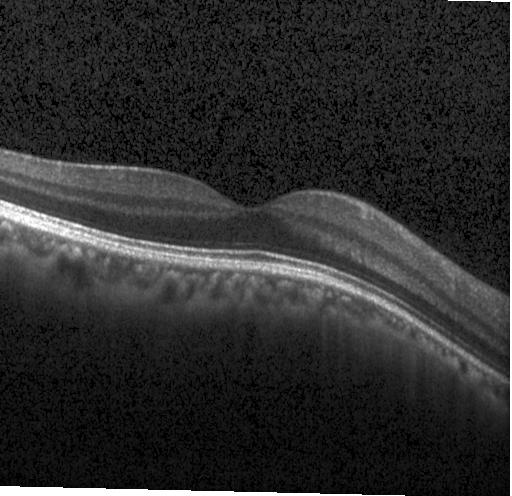
Fovea-centered · spectral-domain optical coherence tomography · OCT B-scan · Heidelberg Spectralis OCT system
Diagnosis: no CNV, DME, or drusen.